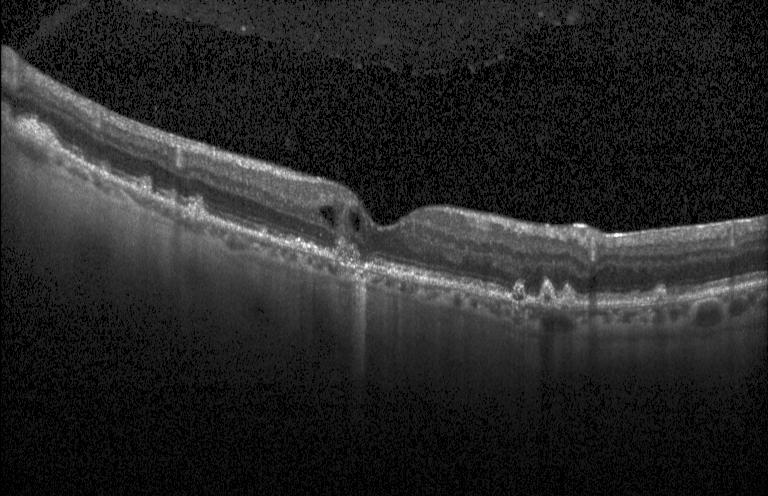
Macular OCT demonstrating a choroidal neovascular membrane.